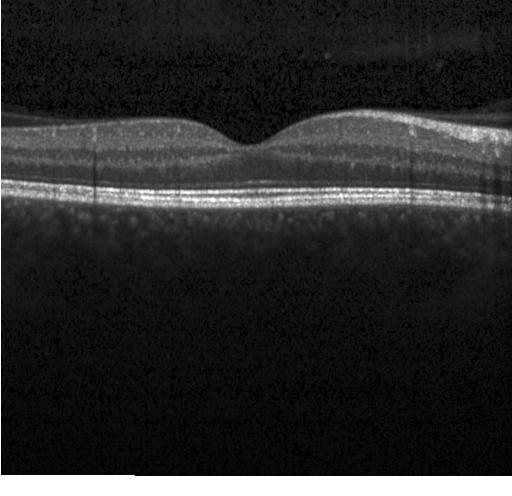 Optical coherence tomography scan. No evidence of choroidal neovascularization, diabetic macular edema, or drusen.